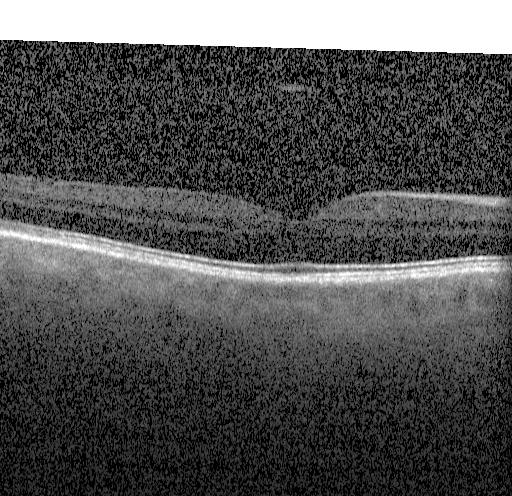 Acquired on a Heidelberg Spectralis, SD-OCT, OCT B-scan, horizontal scan through the fovea.
Macular OCT: no choroidal neovascularization, diabetic macular edema, or drusen.